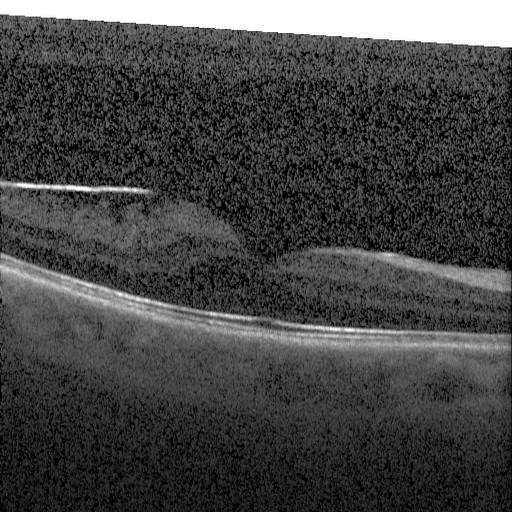

Through the macula; optical coherence tomography B-scan; instrument: Heidelberg Spectralis
Impression: diabetic macular edema.